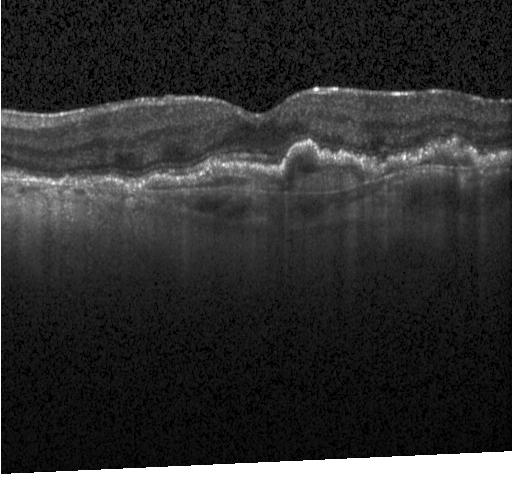 Spectral-domain OCT; OCT line scan.
Finding: a choroidal neovascular membrane.